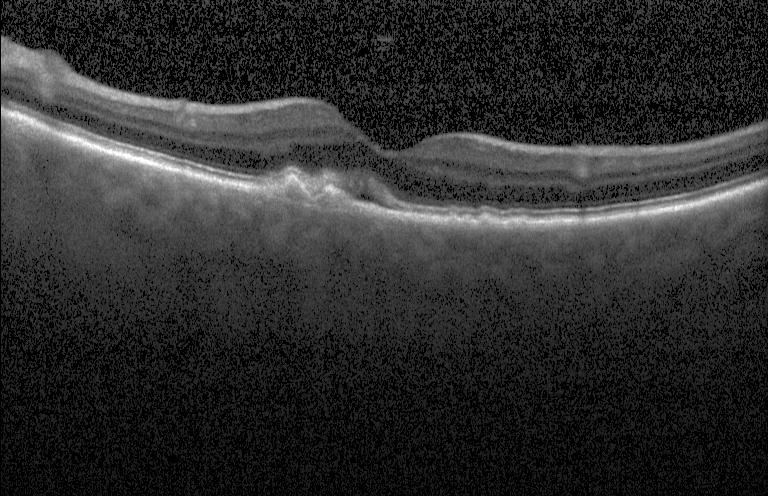
Spectral-domain optical coherence tomography · fovea-centered · retinal OCT cross-section — Finding: a choroidal neovascular membrane.